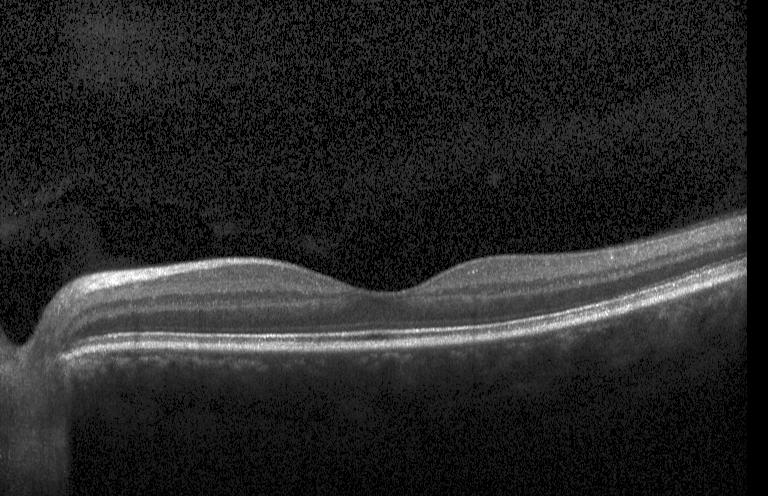

OCT B-scan — Impression: no choroidal neovascularization, diabetic macular edema, or drusen.